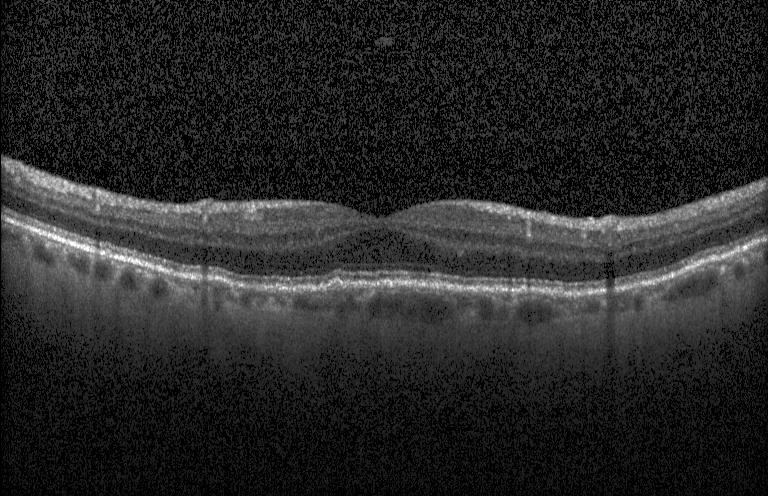
Optical coherence tomography scan
The scan shows multiple drusen.